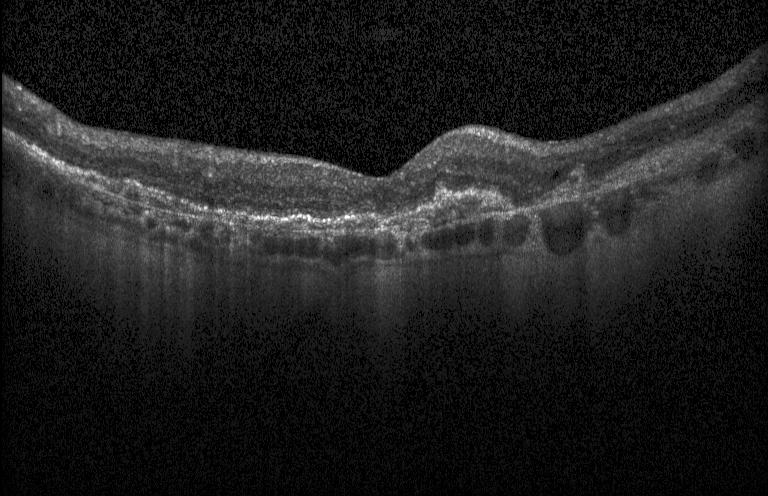

Spectral-domain OCT. Retinal OCT cross-section.
The scan shows a choroidal neovascular membrane.